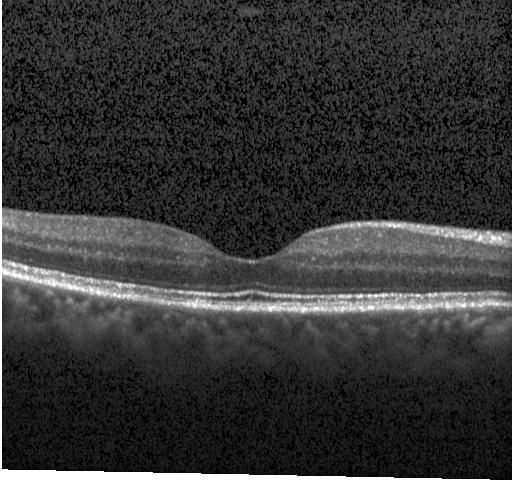 Heidelberg Spectralis; through the macula; spectral-domain OCT; OCT line scan.
This B-scan demonstrates no CNV, no DME, and no drusen.